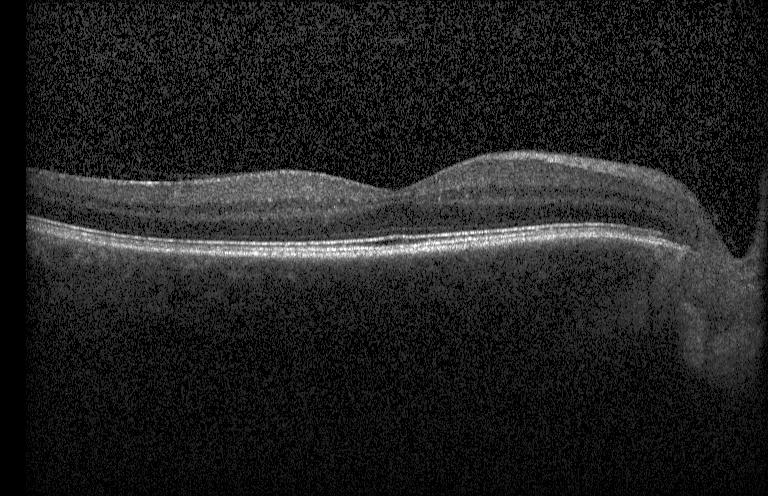

OCT B-scan. Spectral-domain optical coherence tomography. Through the macula. Heidelberg Spectralis OCT system. Finding: neither choroidal neovascularization, diabetic macular edema, nor drusen.